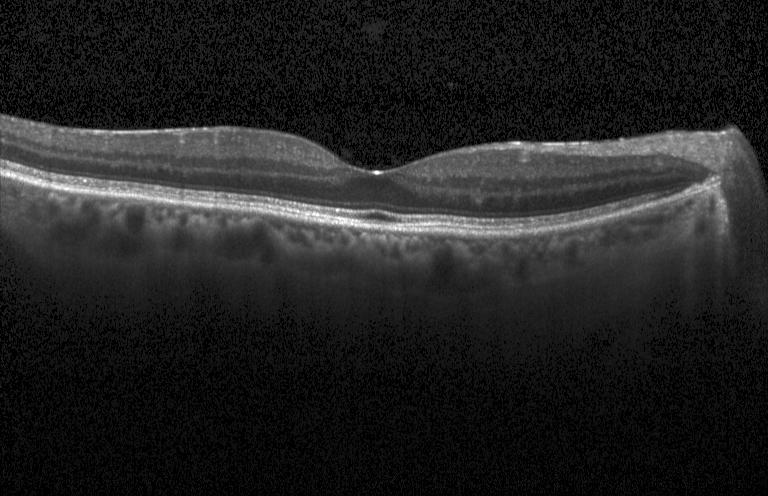

Diagnosis: neither choroidal neovascularization, diabetic macular edema, nor drusen.